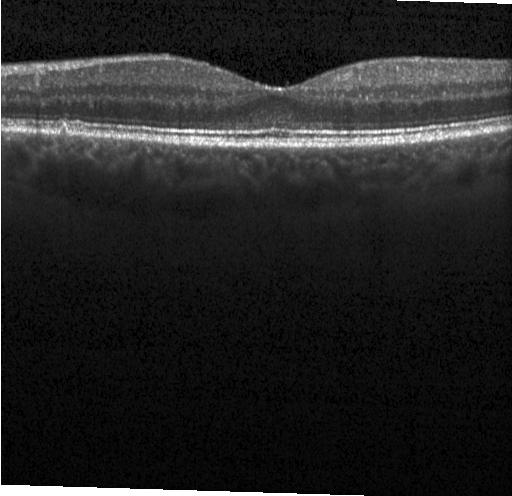
Optical coherence tomography B-scan. This B-scan demonstrates no evidence of CNV, DME, or drusen.